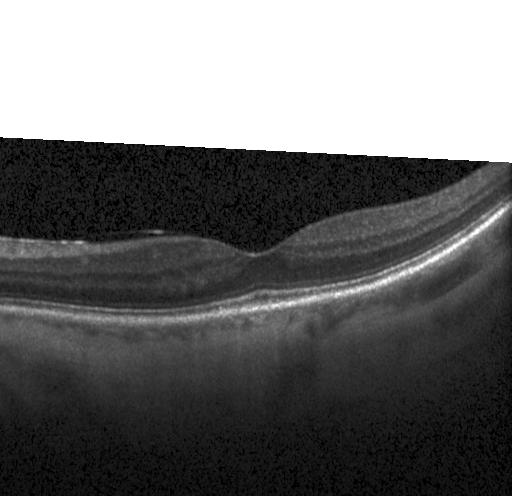

Finding: neither choroidal neovascularization, diabetic macular edema, nor drusen.